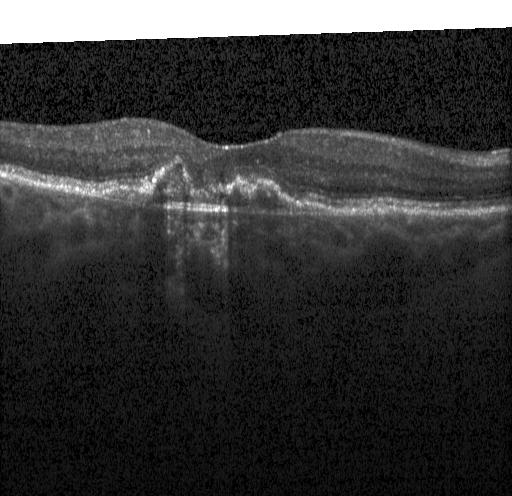

Finding: a choroidal neovascular membrane.